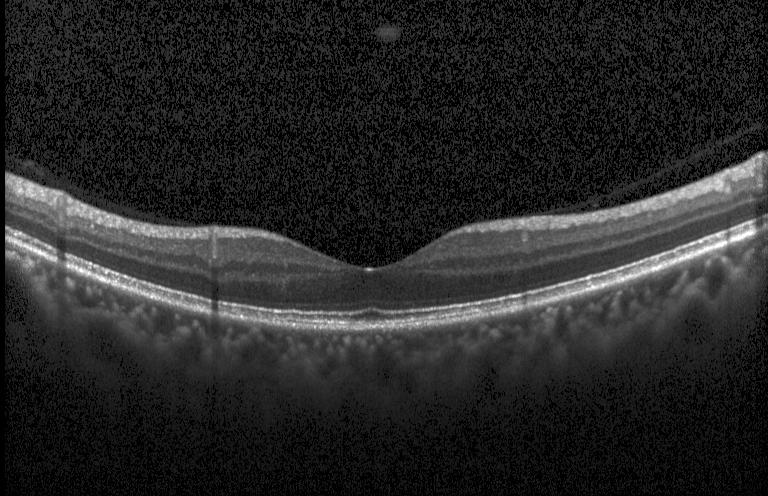 Dx: no evidence of choroidal neovascularization, diabetic macular edema, or drusen.